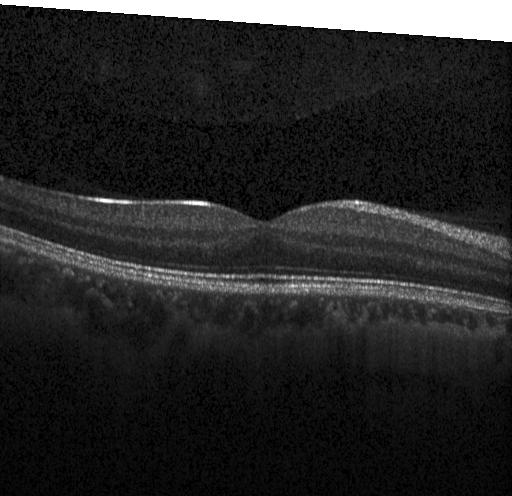

Macular OCT: no choroidal neovascularization, no diabetic macular edema, and no drusen.